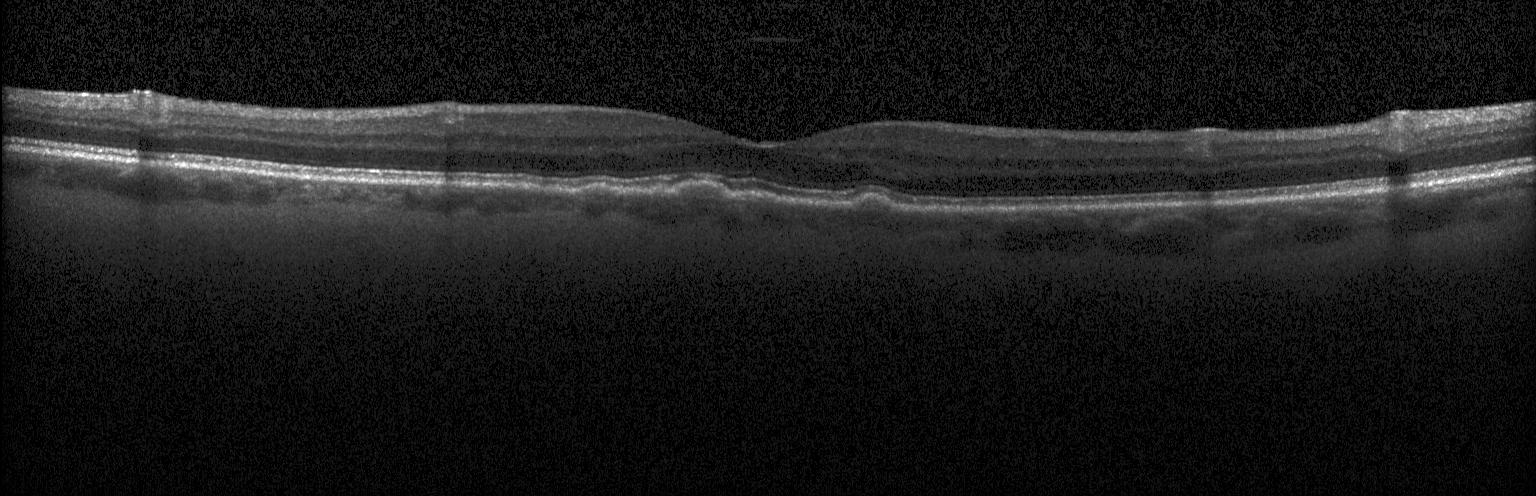 OCT scan showing drusen.